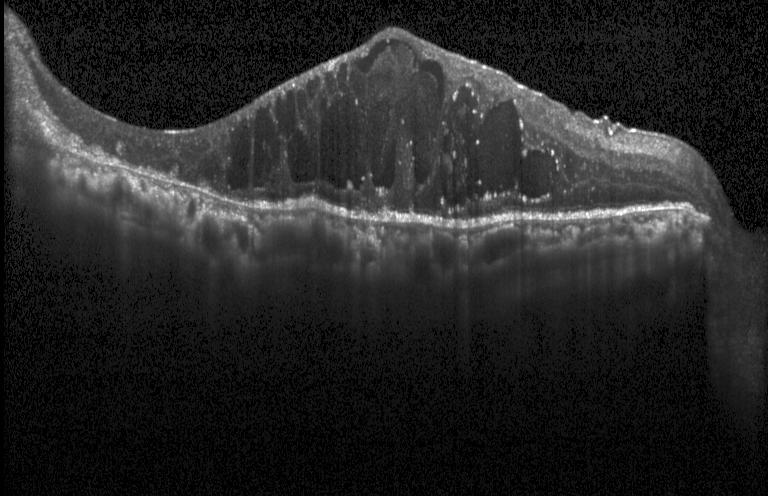

Spectral-domain optical coherence tomography, horizontal scan through the fovea, optical coherence tomography B-scan. Impression: diabetic macular edema (DME).